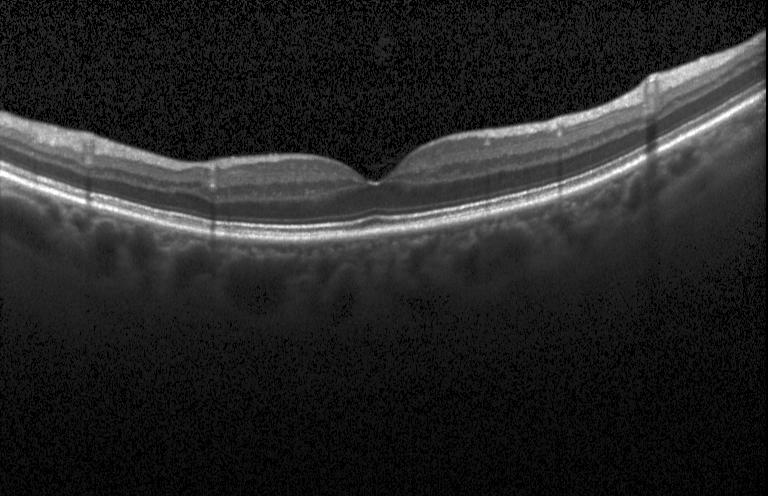

Spectral-domain optical coherence tomography. Heidelberg Spectralis OCT system. Retinal OCT B-scan. Centered on the fovea
Diagnosis: no evidence of choroidal neovascularization, diabetic macular edema, or drusen.